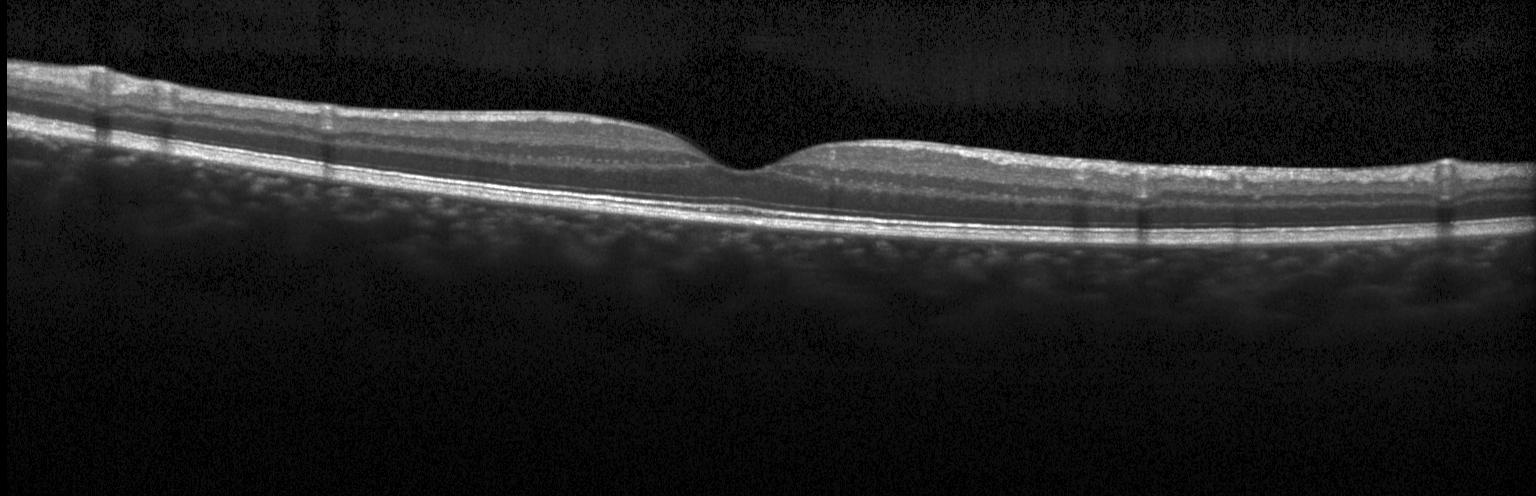

Impression: no choroidal neovascularization, diabetic macular edema, or drusen.